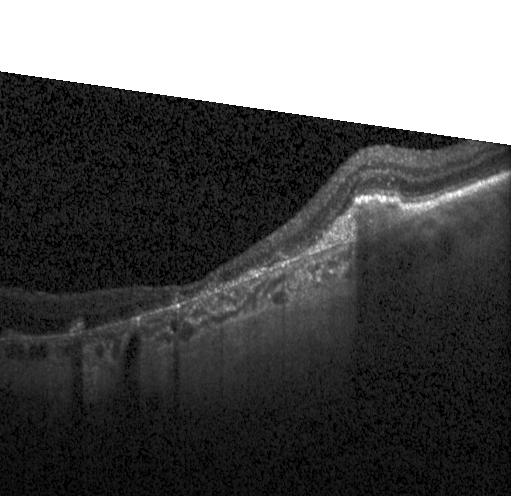

The scan shows choroidal neovascularization.